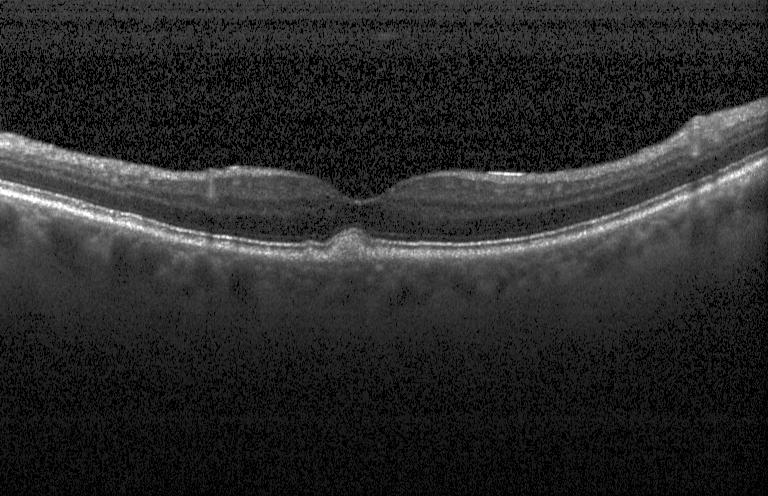
Spectral-domain OCT; OCT line scan; instrument: Heidelberg Spectralis; fovea-centered
Dx: multiple drusen.